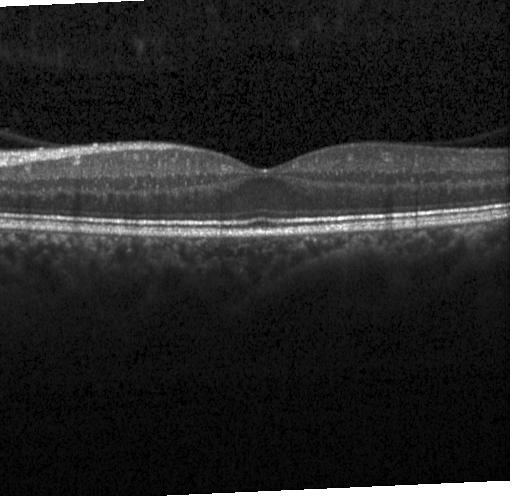 OCT B-scan. Horizontal scan through the fovea — Macular OCT: no choroidal neovascularization, no diabetic macular edema, and no drusen.